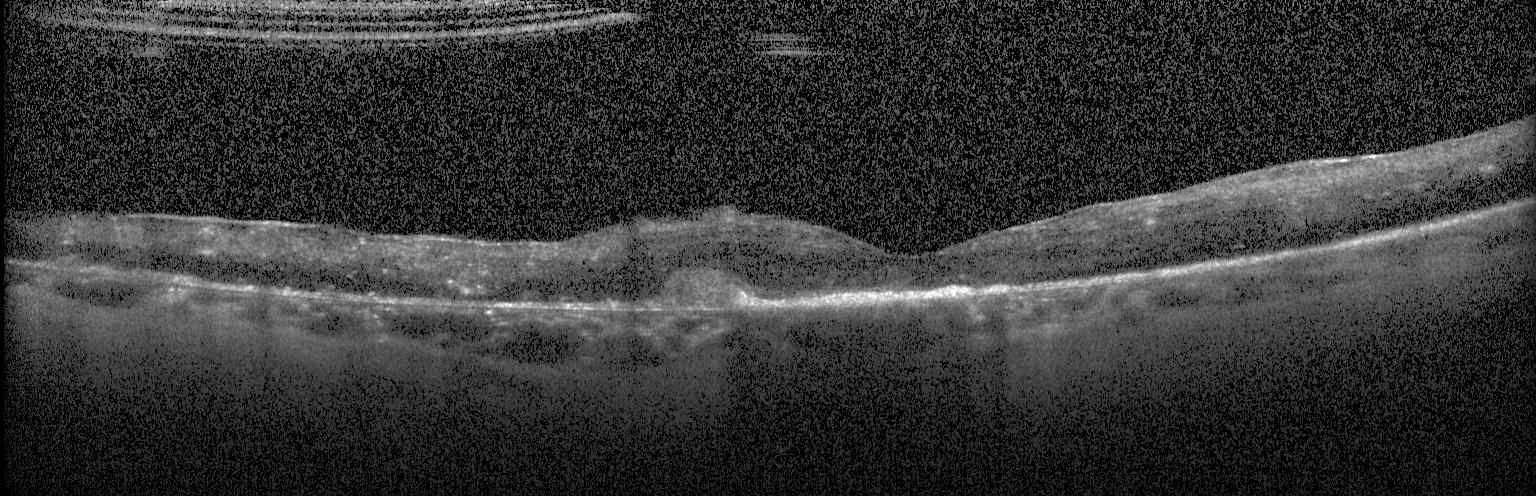

Spectral-domain OCT B-scan: a choroidal neovascular membrane.